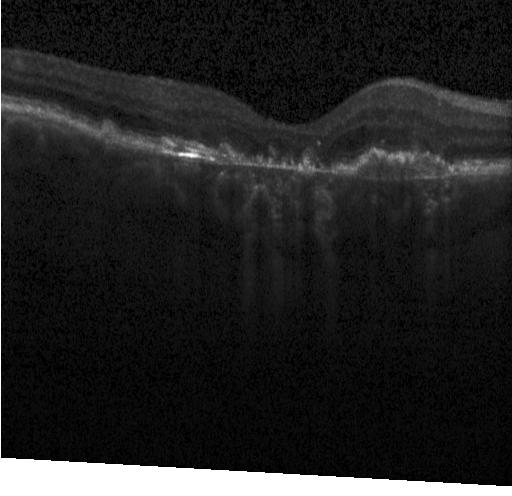

Macular OCT demonstrating choroidal neovascularization (CNV).